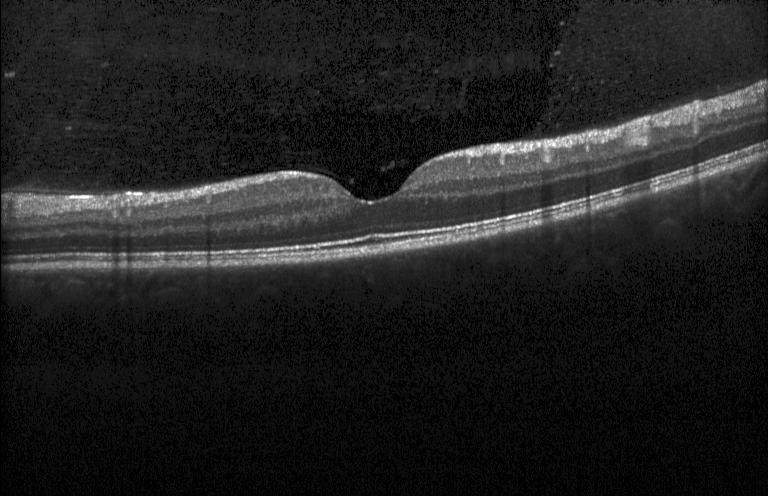 Retinal OCT B-scan.
Macular OCT: neither CNV, DME, nor drusen.